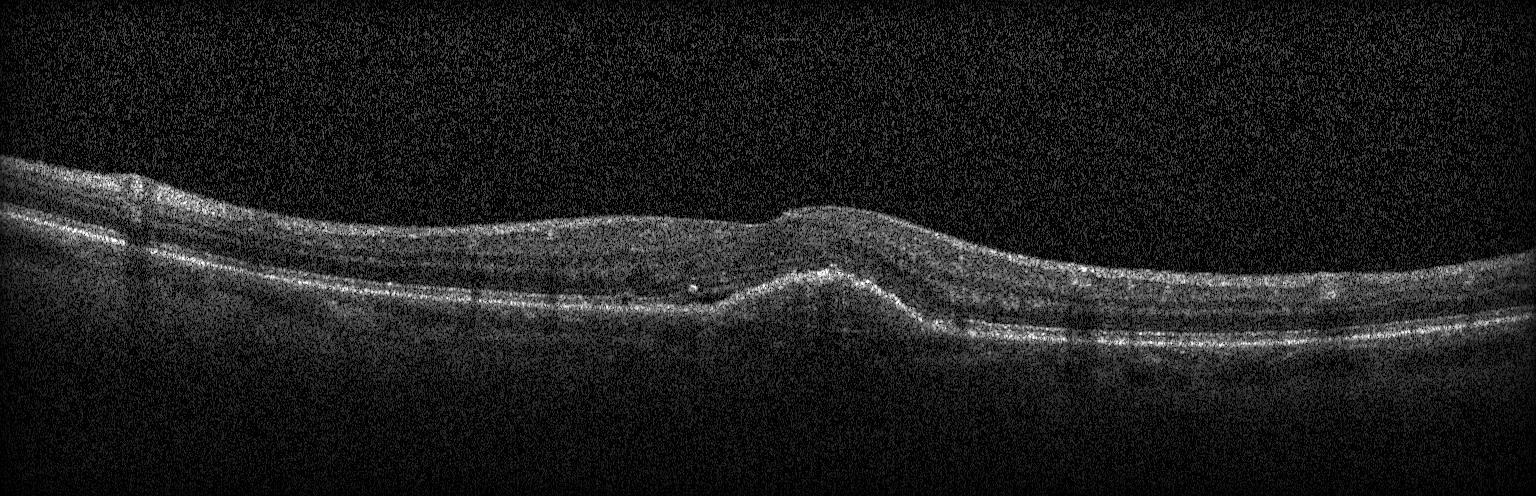 Diagnosis: a choroidal neovascular membrane.